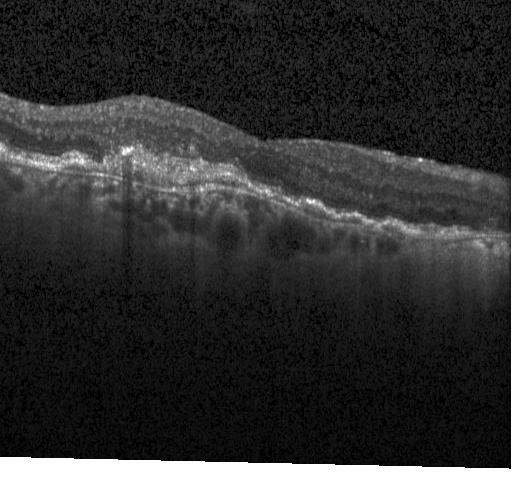

OCT finding: CNV.